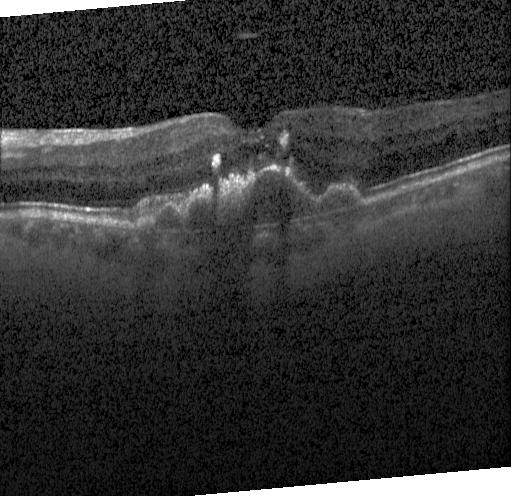

OCT line scan
OCT finding: a choroidal neovascular membrane.